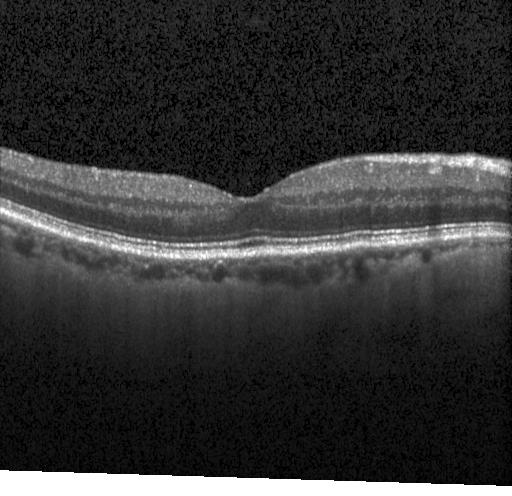 Through the macula, retinal OCT cross-section, acquired on a Heidelberg Spectralis. Diagnosis: neither choroidal neovascularization, diabetic macular edema, nor drusen.